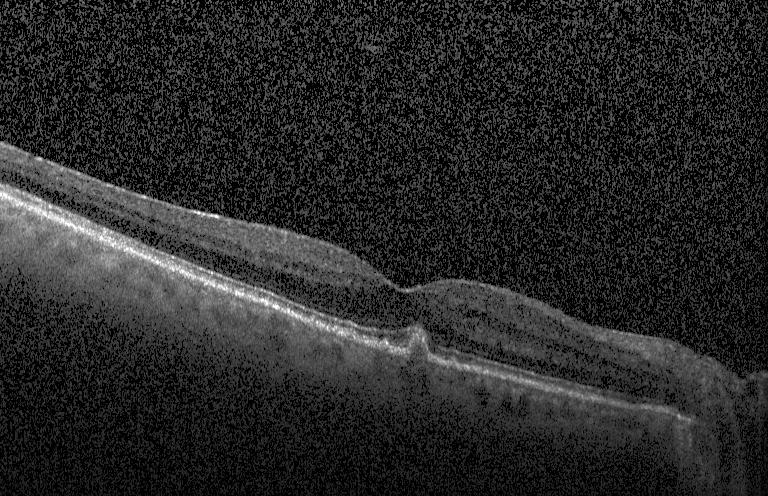

OCT line scan. Spectral-domain OCT. Heidelberg Spectralis OCT system. Macular scan.
OCT finding: sub-RPE drusenoid deposits.